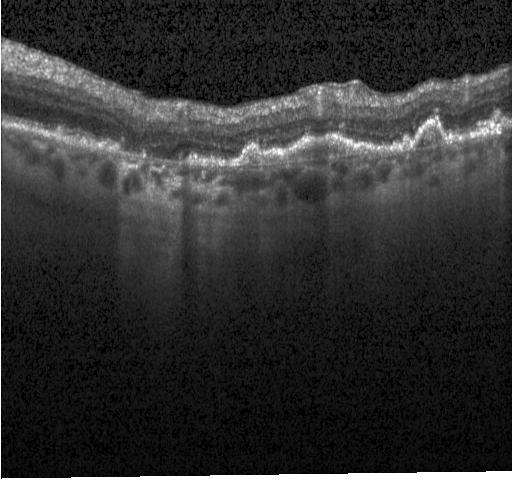

Finding: choroidal neovascularization (CNV).